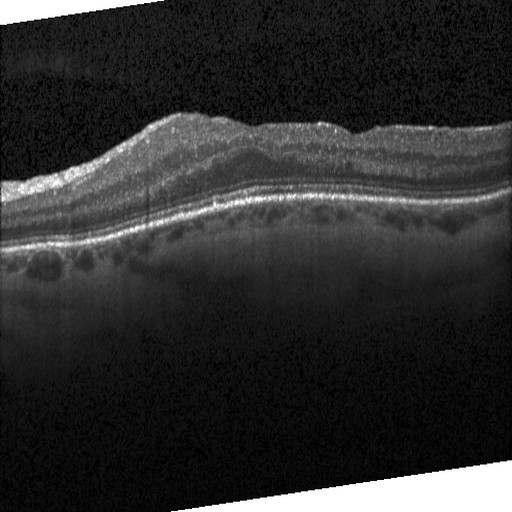 Finding: diabetic macular edema (DME).